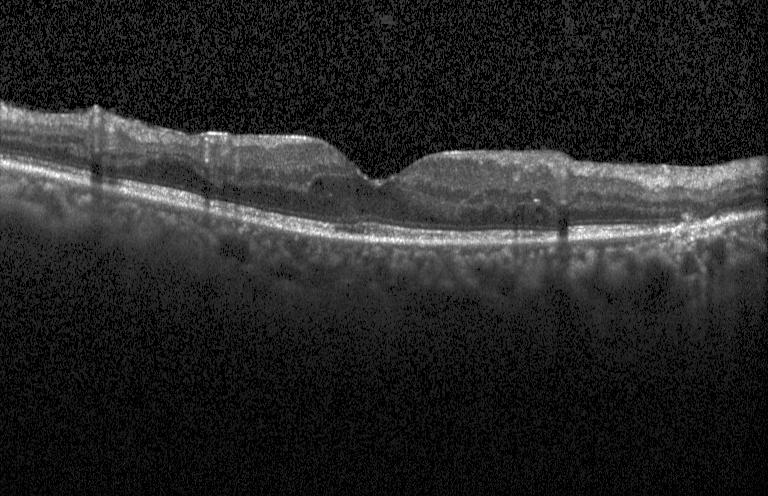 Retinal OCT cross-section showing diabetic macular edema.